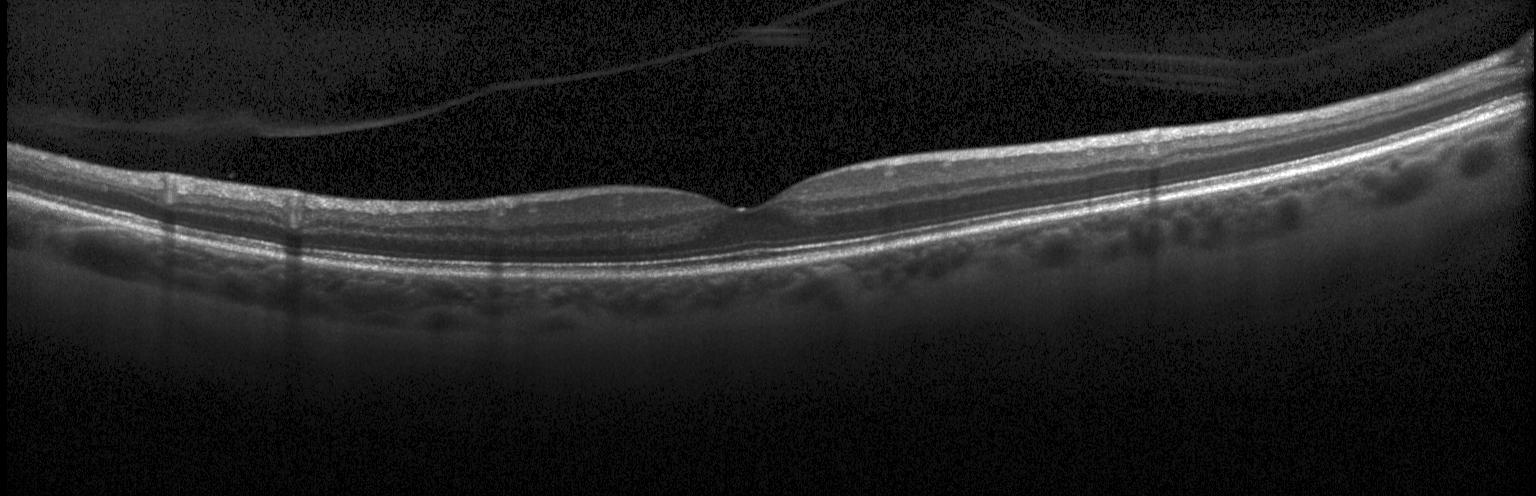 Optical coherence tomography scan — Impression: no choroidal neovascularization, diabetic macular edema, or drusen.